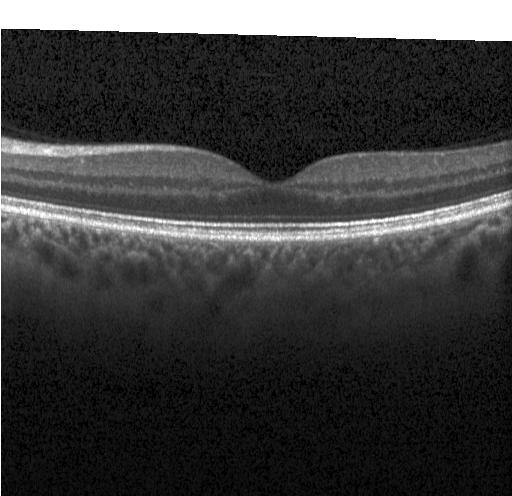
OCT line scan; spectral-domain OCT
Assessment: neither choroidal neovascularization, diabetic macular edema, nor drusen.